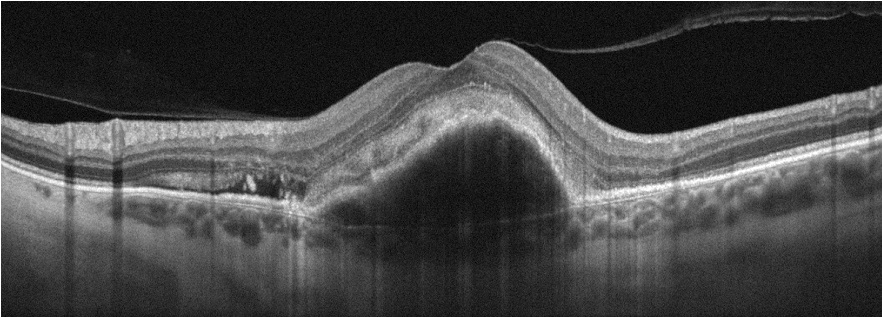

Optovue Avanti RTVue XR; optical coherence tomography scan; fovea-centered. Diagnosis: age-related macular degeneration.